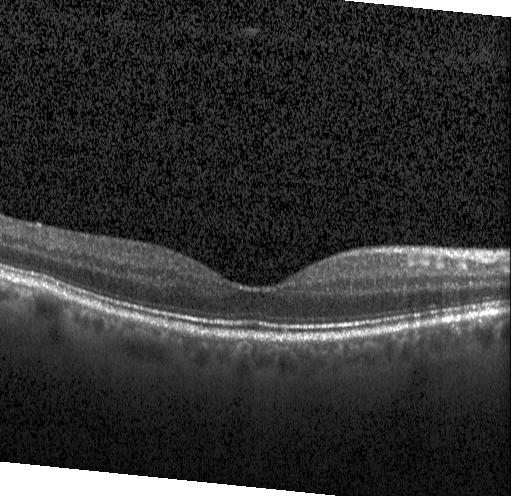

Optical coherence tomography scan · Heidelberg Spectralis · horizontal scan through the fovea. Assessment: no evidence of CNV, DME, or drusen.